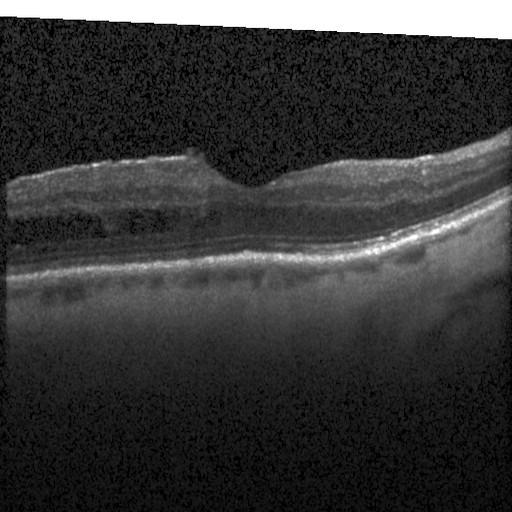
Impression: diabetic macular edema.